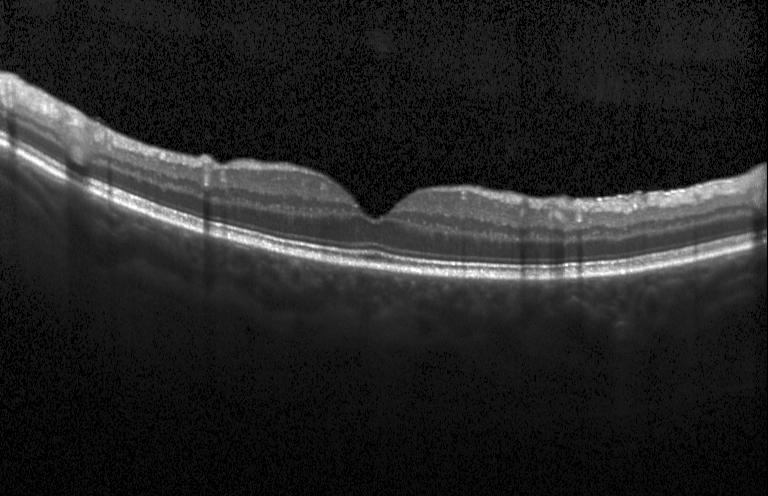

Macular OCT: no CNV, DME, or drusen.